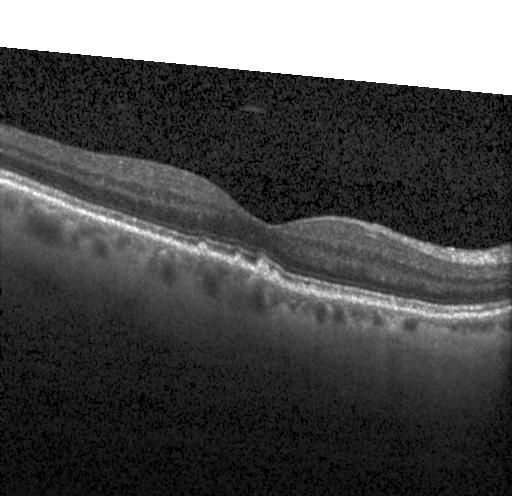 OCT line scan
Diagnosis: multiple drusen.